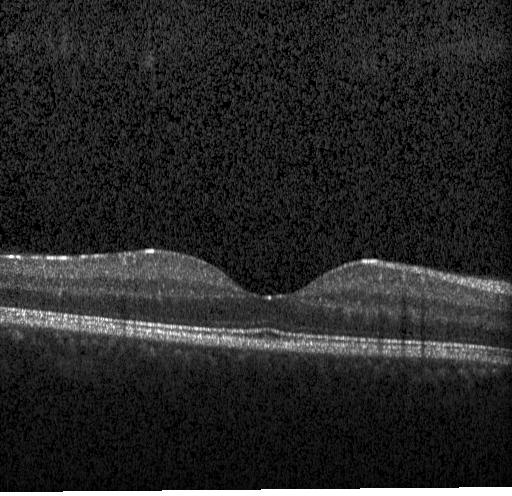
Finding: no choroidal neovascularization, no diabetic macular edema, and no drusen.